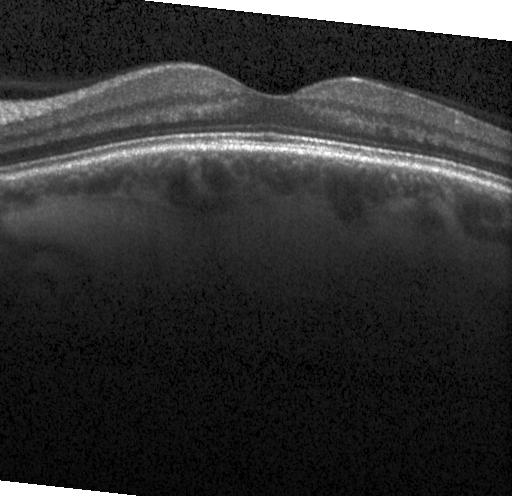

Heidelberg Spectralis OCT system, spectral-domain optical coherence tomography, horizontal scan through the fovea, retinal OCT B-scan.
Impression: no choroidal neovascularization, no diabetic macular edema, and no drusen.